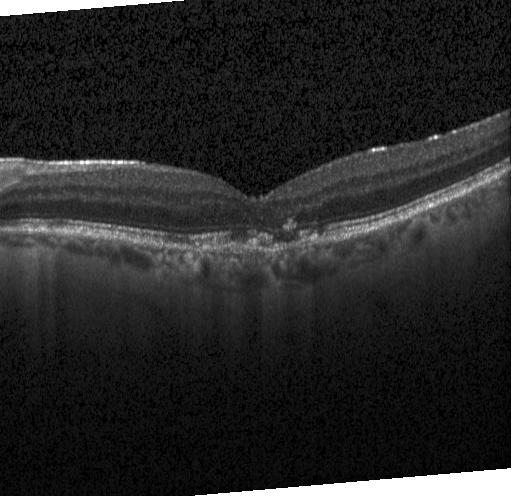
Retinal OCT B-scan — Finding: choroidal neovascularization.